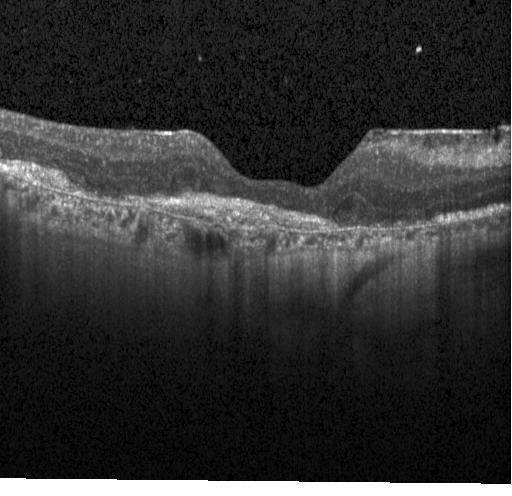 Retinal OCT B-scan — Impression: a choroidal neovascular membrane.